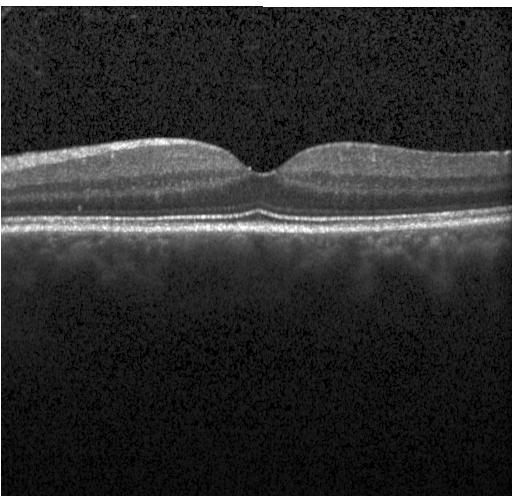

Acquired on a Heidelberg Spectralis; fovea-centered; retinal OCT B-scan — Finding: neither CNV, DME, nor drusen.